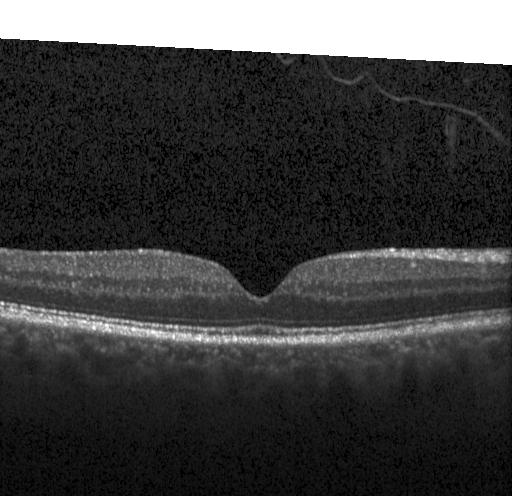
SD-OCT; through the macula; retinal OCT B-scan
This B-scan demonstrates no choroidal neovascularization, diabetic macular edema, or drusen.